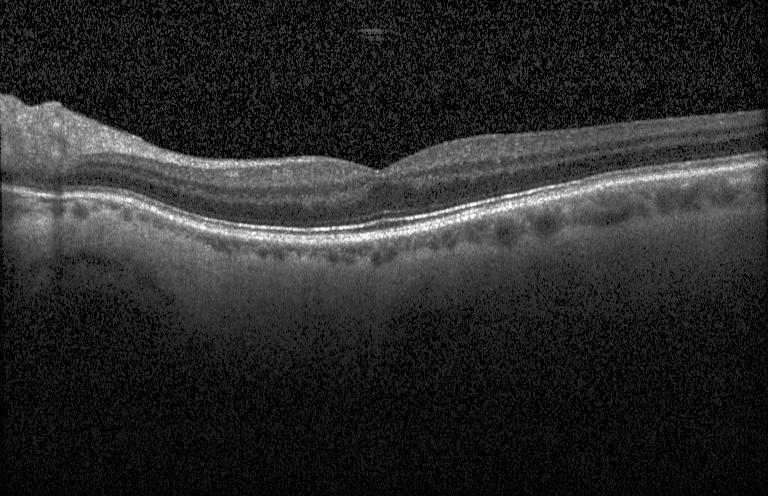 Diagnosis: neither CNV, DME, nor drusen.